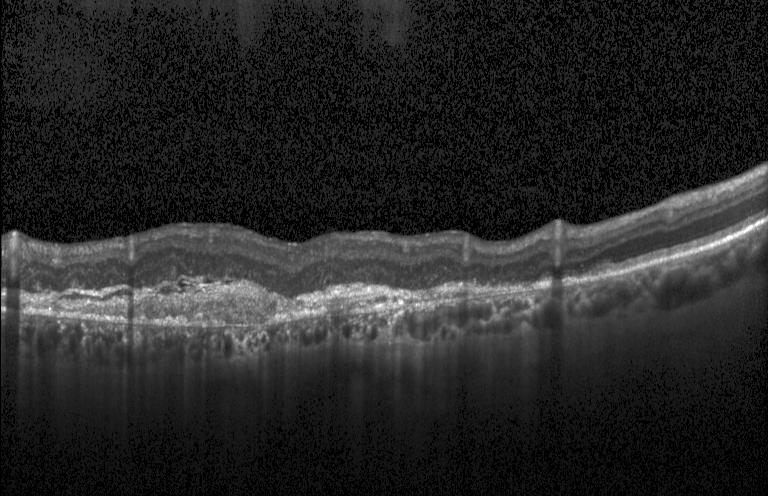
Assessment: choroidal neovascularization.